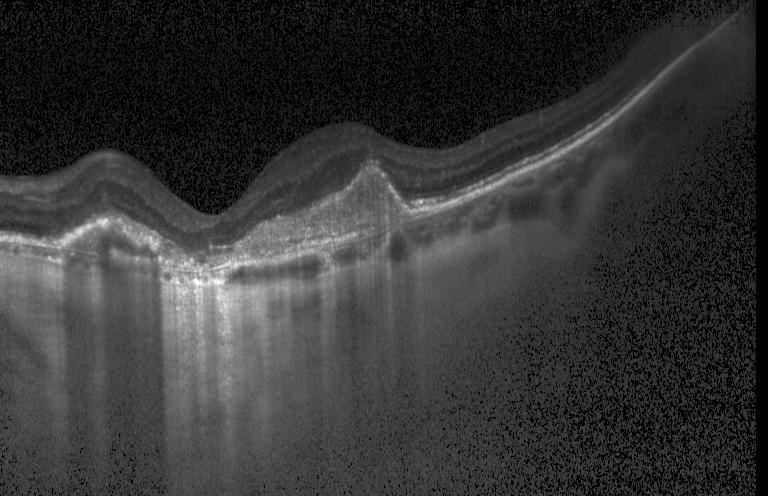 Retinal OCT cross-section. Spectral-domain OCT. The scan shows choroidal neovascularization (CNV).